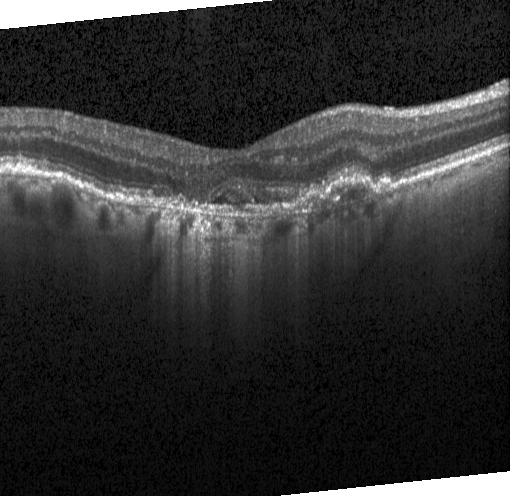 This B-scan demonstrates choroidal neovascularization (CNV).